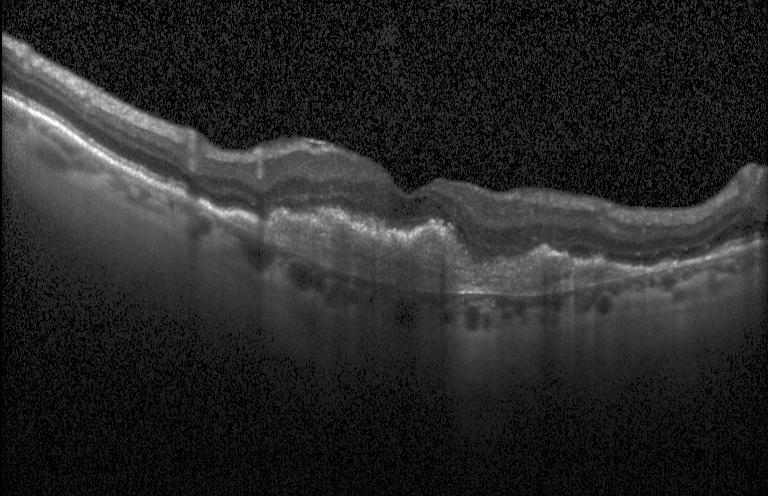
Optical coherence tomography B-scan. Spectral-domain OCT. Macular scan. Heidelberg Spectralis.
Impression: choroidal neovascularization.